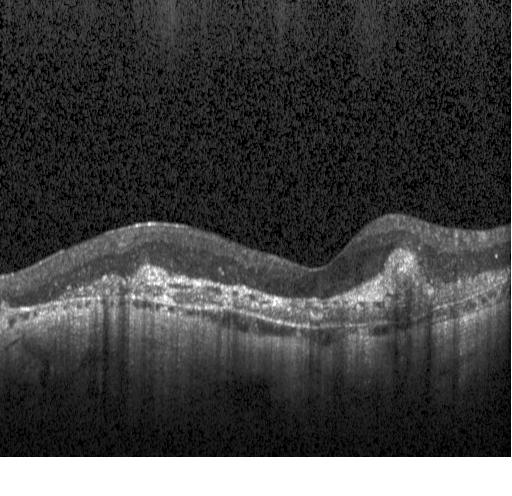

A choroidal neovascular membrane.